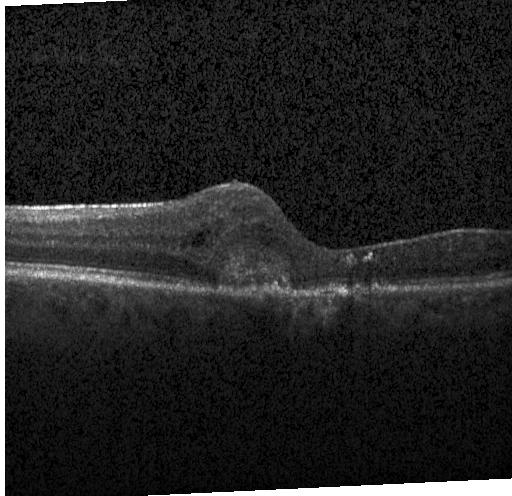

OCT line scan · spectral-domain OCT · instrument: Heidelberg Spectralis.
This B-scan demonstrates choroidal neovascularization.